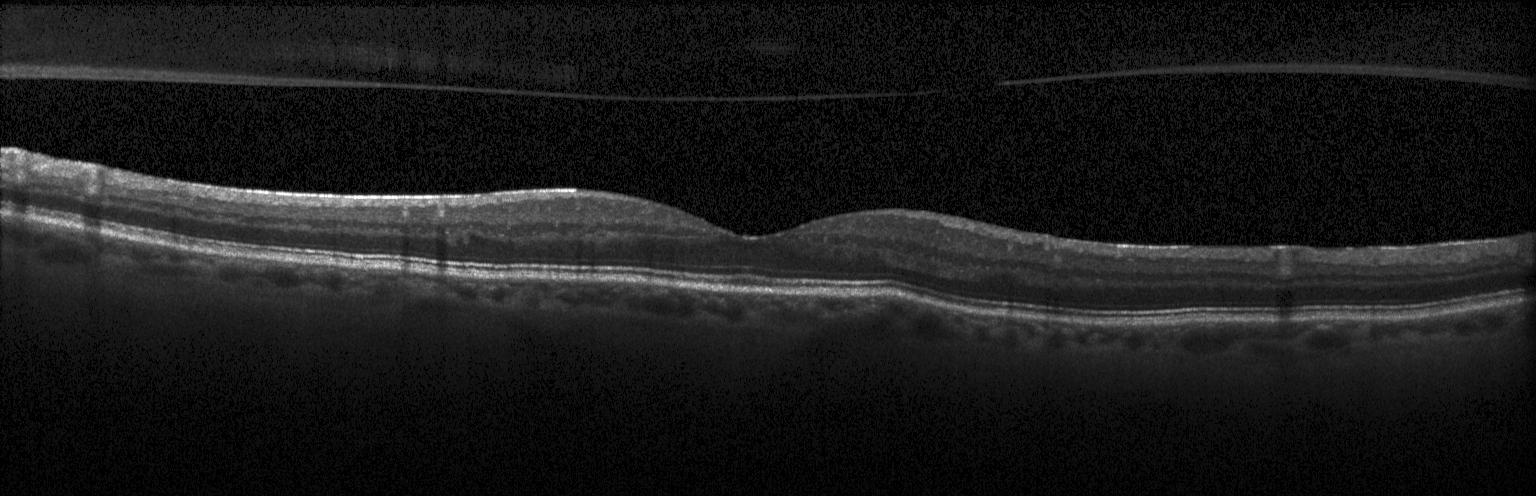
Impression: no evidence of choroidal neovascularization, diabetic macular edema, or drusen.